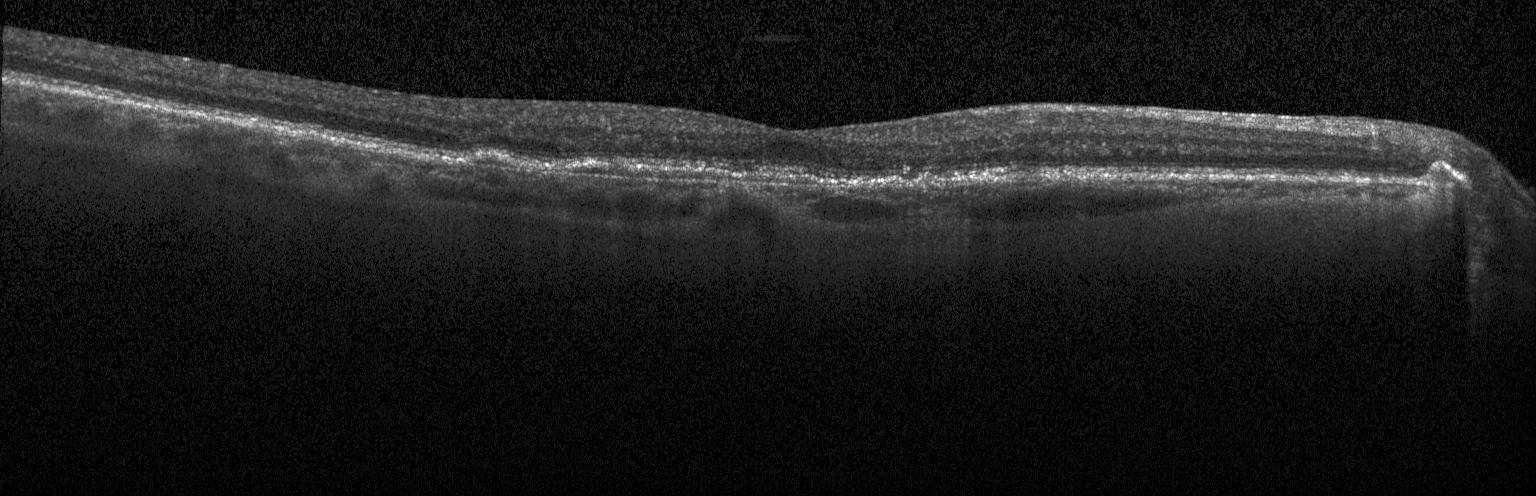
Through the macula, optical coherence tomography B-scan. Assessment: a choroidal neovascular membrane.